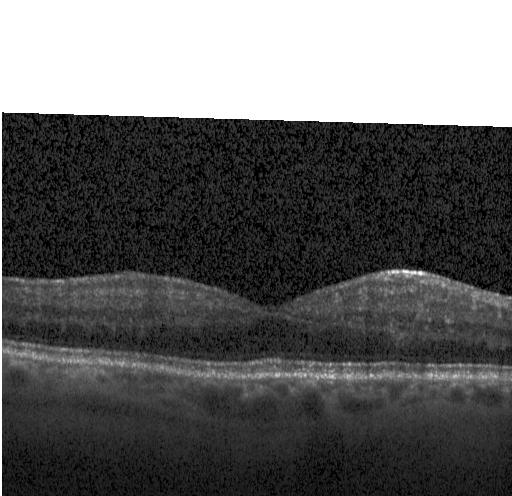
Finding: no choroidal neovascularization, no diabetic macular edema, and no drusen.